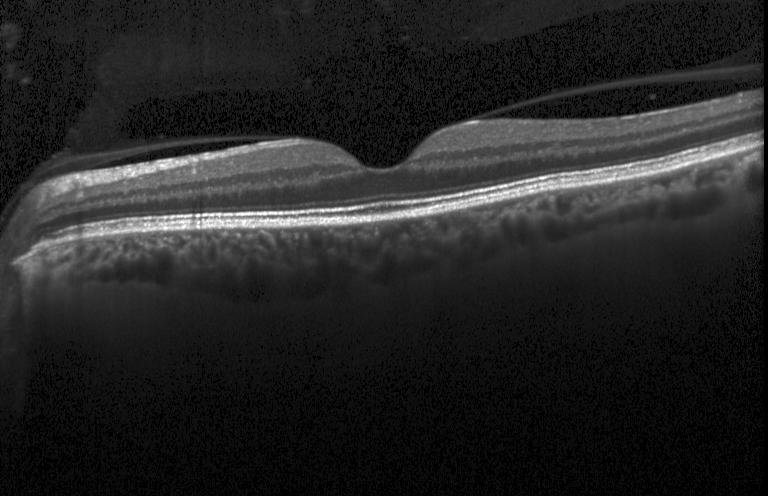 Macular scan, OCT B-scan. Diagnosis: no choroidal neovascularization, diabetic macular edema, or drusen.